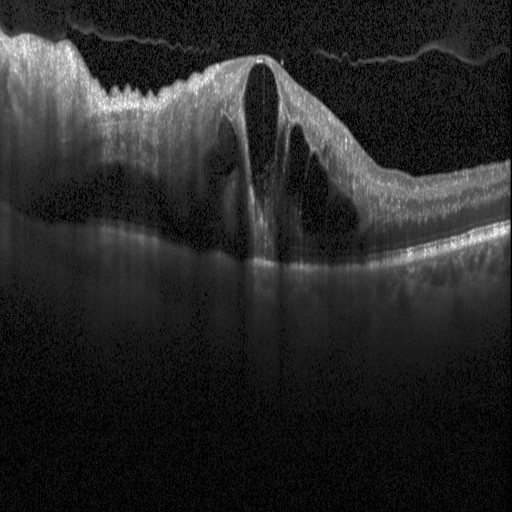
Diagnosis: diabetic macular edema.